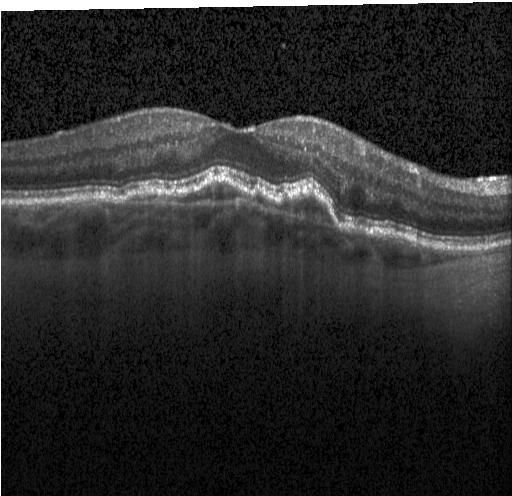
Macular OCT: CNV.